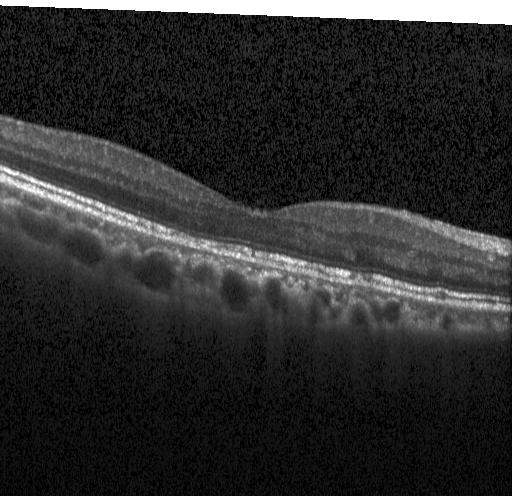
Heidelberg Spectralis OCT system. OCT B-scan. Through the macula. SD-OCT — Diagnosis: no evidence of choroidal neovascularization, diabetic macular edema, or drusen.